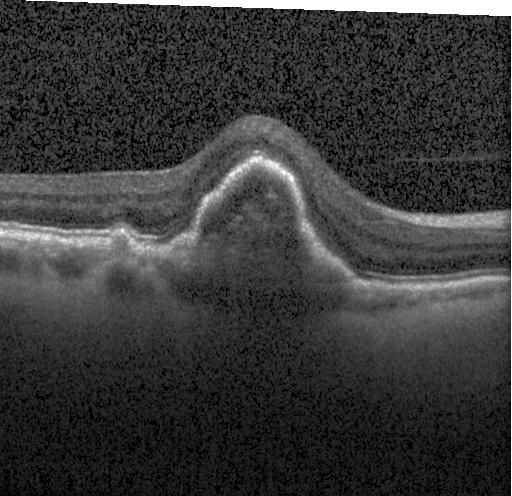

OCT line scan — Choroidal neovascularization.